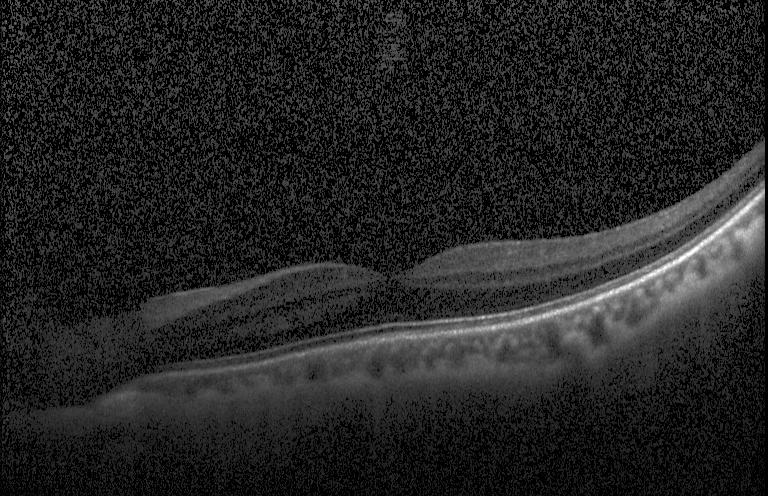 Dx: no CNV, no DME, and no drusen.